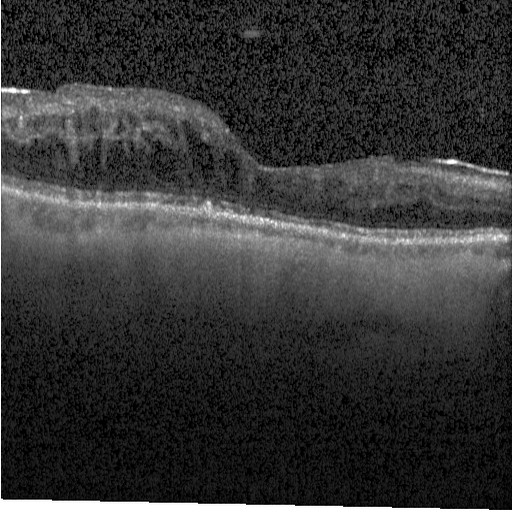

Heidelberg Spectralis. OCT line scan. Spectral-domain OCT. Horizontal scan through the fovea. Diagnosis: diabetic macular edema (DME).